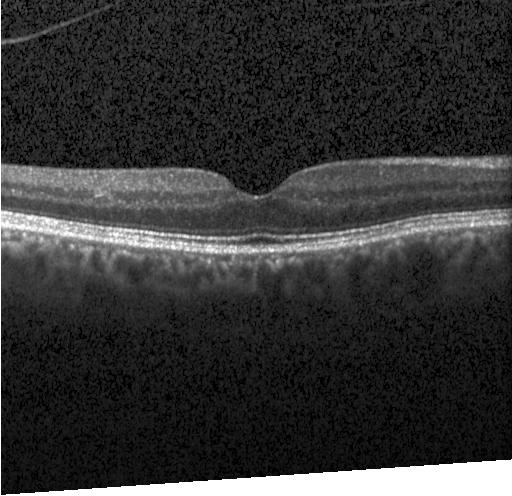 OCT line scan · instrument: Heidelberg Spectralis — Assessment: no CNV, DME, or drusen.